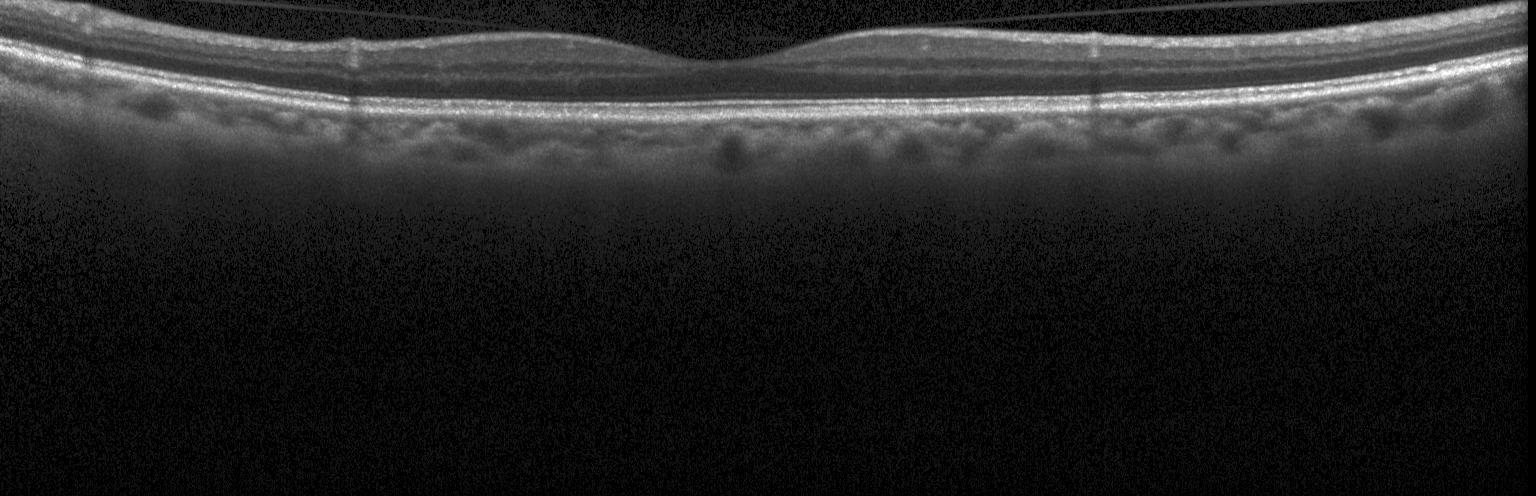
Macular OCT: neither CNV, DME, nor drusen.